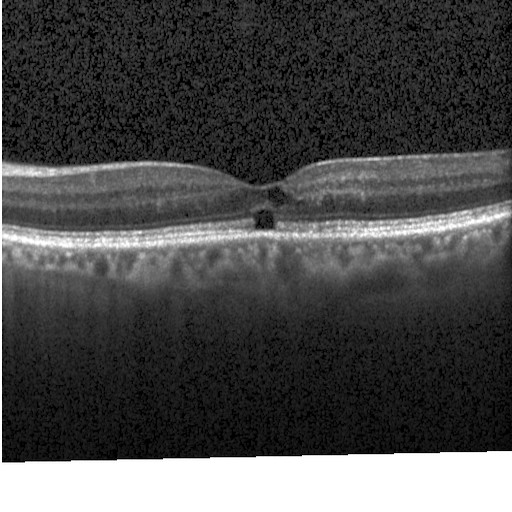
OCT B-scan, acquired on a Heidelberg Spectralis.
Macular OCT: diabetic macular edema (DME).